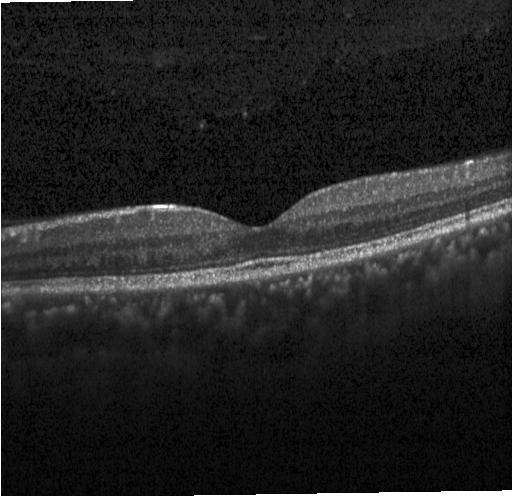
Retinal OCT cross-section. Macular scan
Impression: neither CNV, DME, nor drusen.